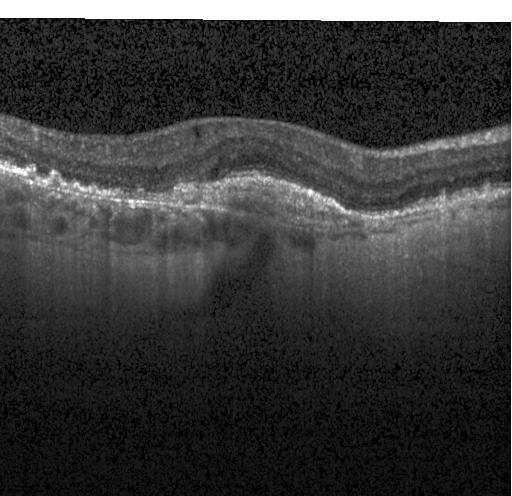 Assessment: choroidal neovascularization (CNV).